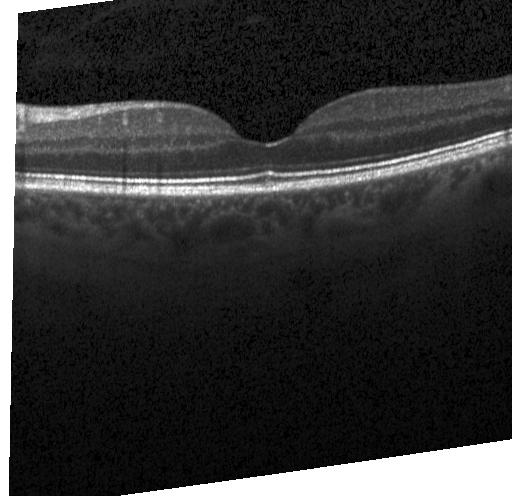 OCT B-scan. Impression: no choroidal neovascularization, no diabetic macular edema, and no drusen.